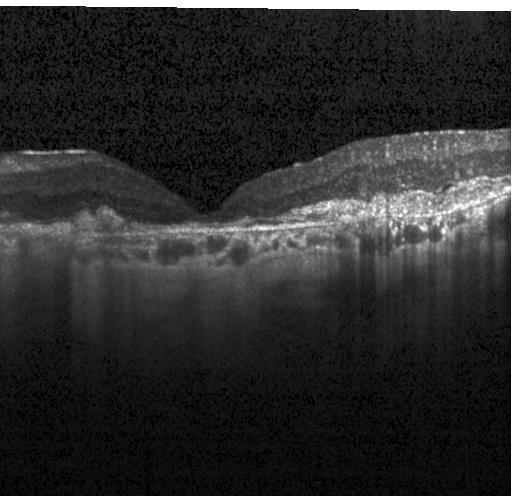 Optical coherence tomography B-scan — Finding: choroidal neovascularization (CNV).